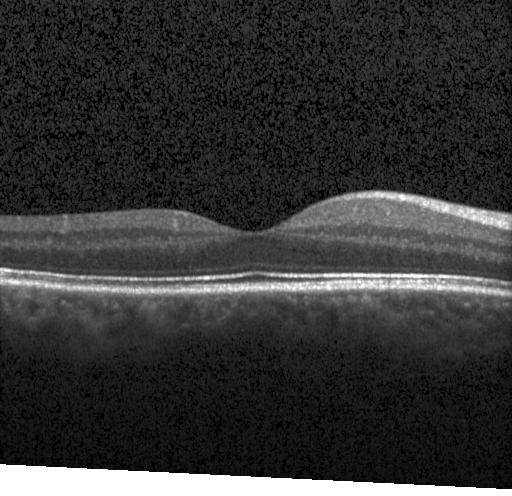
OCT B-scan showing no CNV, no DME, and no drusen.